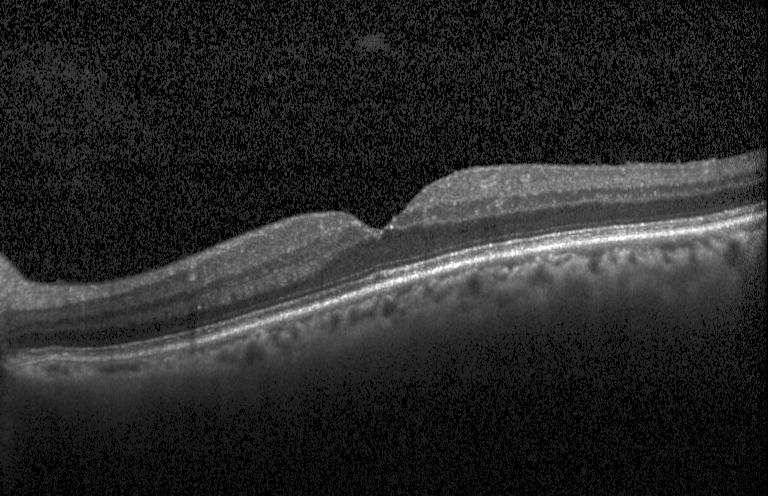

Spectral-domain OCT, macular scan, OCT line scan
Finding: neither choroidal neovascularization, diabetic macular edema, nor drusen.